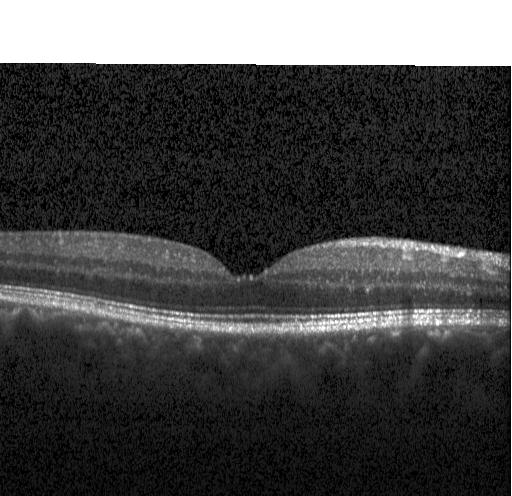
Spectral-domain OCT · retinal OCT cross-section · Heidelberg Spectralis OCT system · fovea-centered. Dx: no evidence of CNV, DME, or drusen.